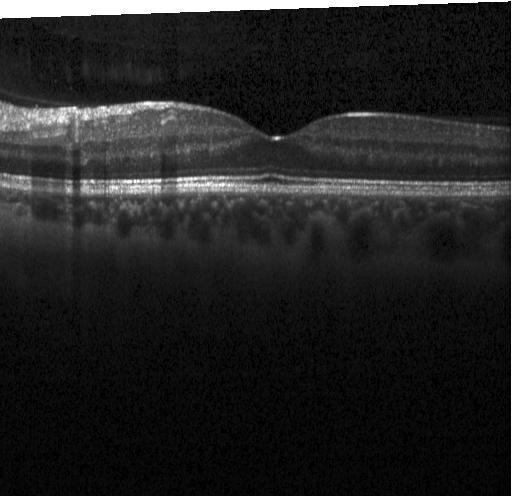 OCT B-scan, Heidelberg Spectralis OCT system — Impression: no evidence of choroidal neovascularization, diabetic macular edema, or drusen.